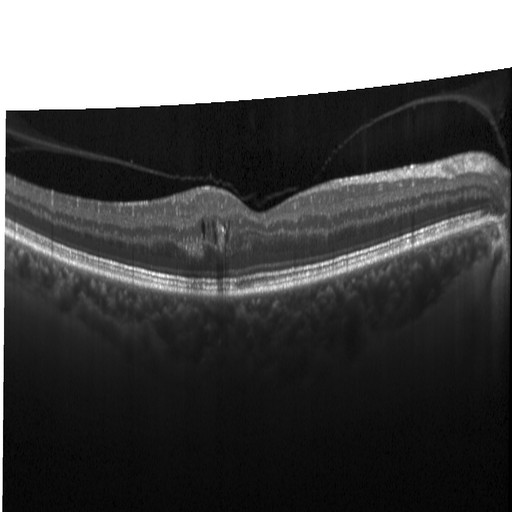
SD-OCT, optical coherence tomography scan. This B-scan demonstrates diabetic macular edema (DME).